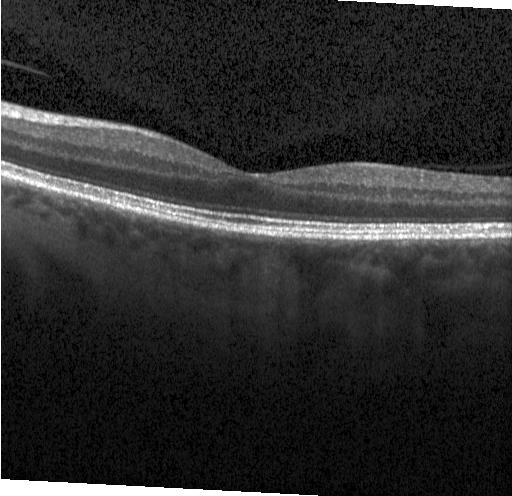
Retinal OCT cross-section — Diagnosis: no evidence of choroidal neovascularization, diabetic macular edema, or drusen.